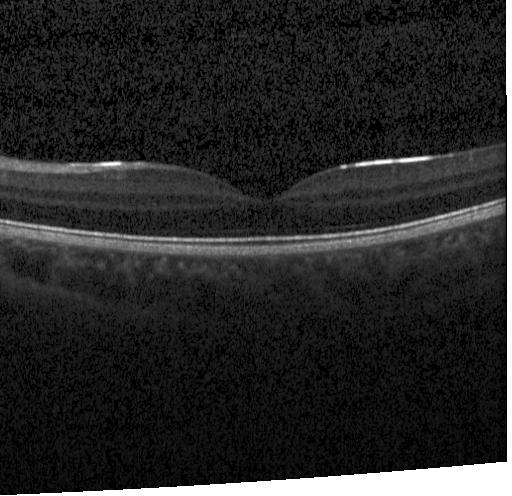 Macular OCT: no choroidal neovascularization, diabetic macular edema, or drusen.